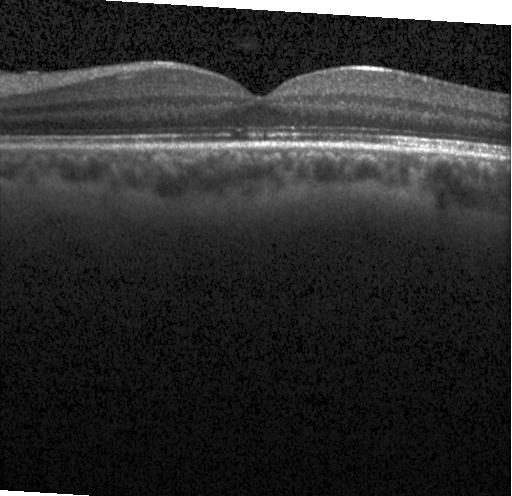

Spectral-domain OCT, retinal OCT B-scan, horizontal scan through the fovea, acquired on a Heidelberg Spectralis — This B-scan demonstrates neither choroidal neovascularization, diabetic macular edema, nor drusen.